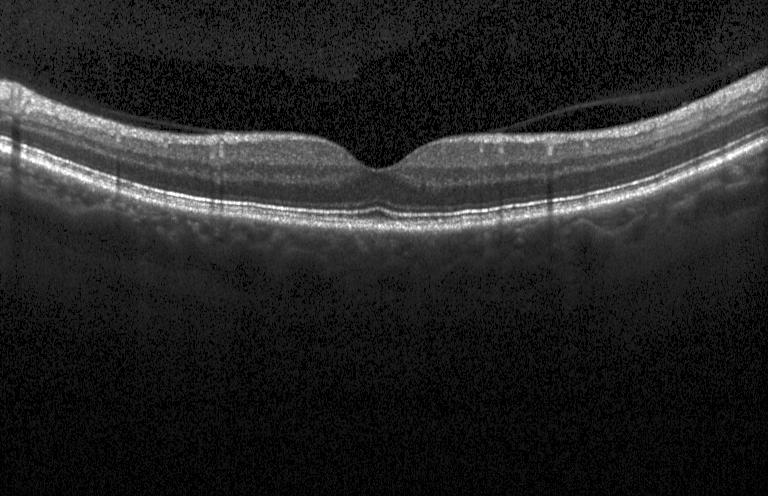
Acquired on a Heidelberg Spectralis, optical coherence tomography B-scan — Assessment: neither choroidal neovascularization, diabetic macular edema, nor drusen.